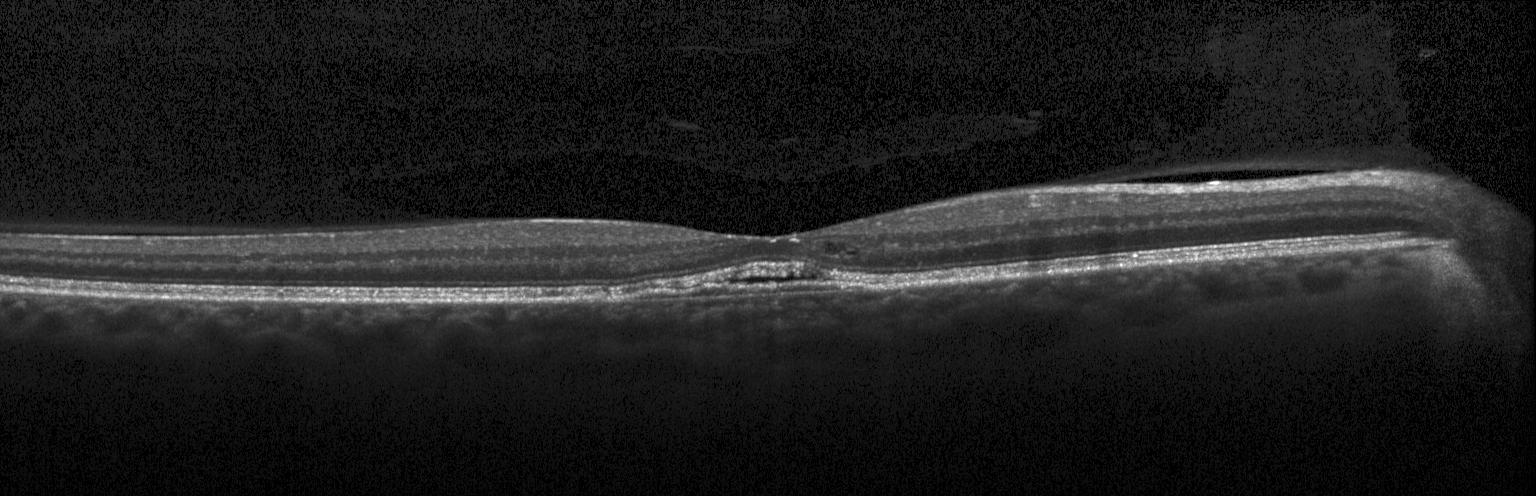 SD-OCT · OCT B-scan.
Finding: a choroidal neovascular membrane.